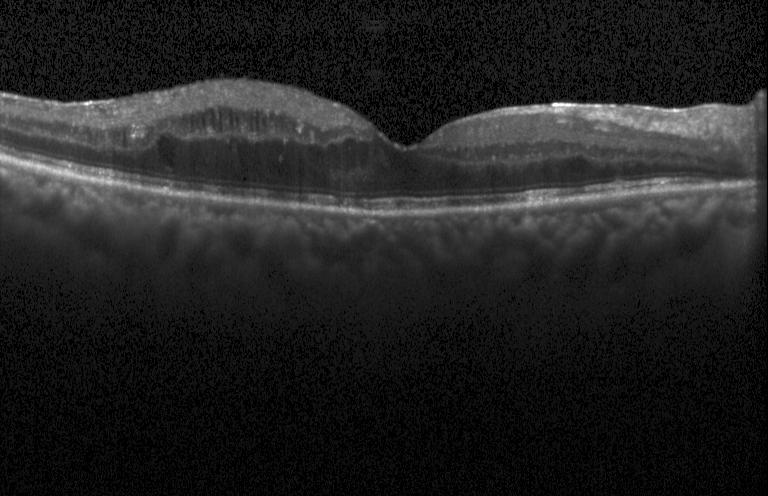 Horizontal scan through the fovea, optical coherence tomography scan — DME.